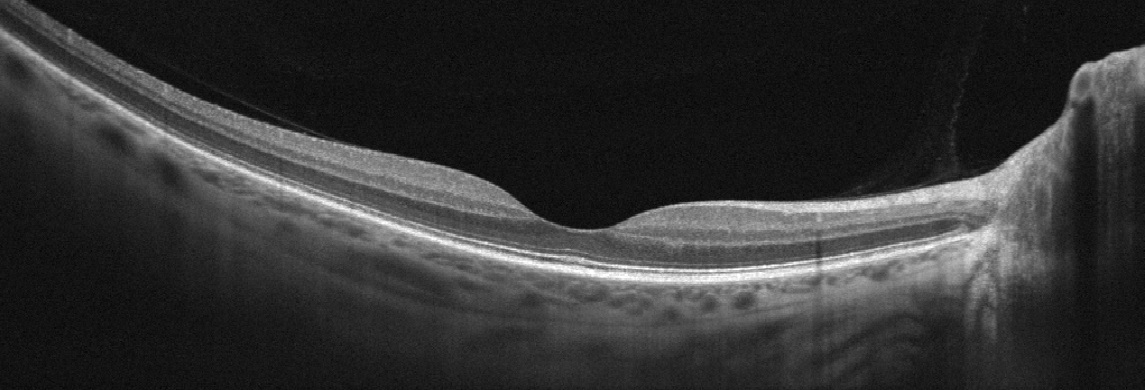 Optical coherence tomography scan; Optovue Avanti RTVue XR. Assessment: no evidence of AMD, DME, ERM, RAO, RVO, or VID.